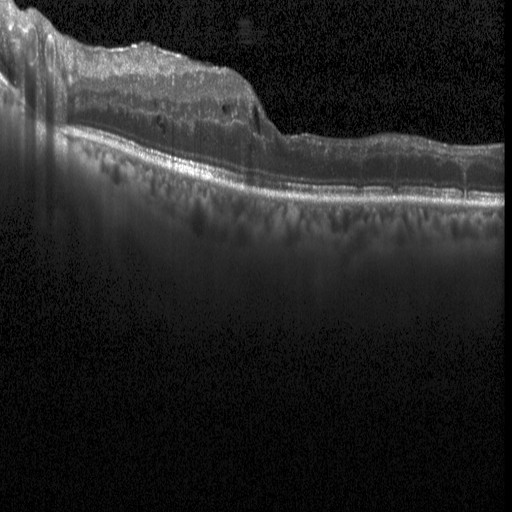
OCT finding: DME.